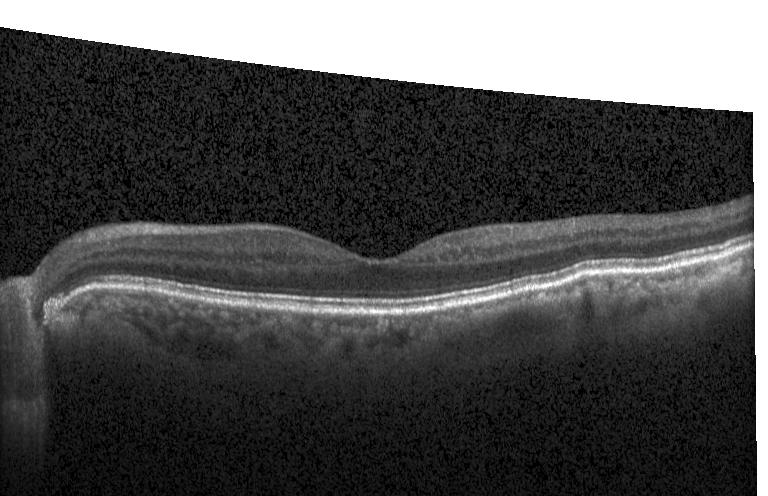
Retinal OCT B-scan — Assessment: no choroidal neovascularization, no diabetic macular edema, and no drusen.